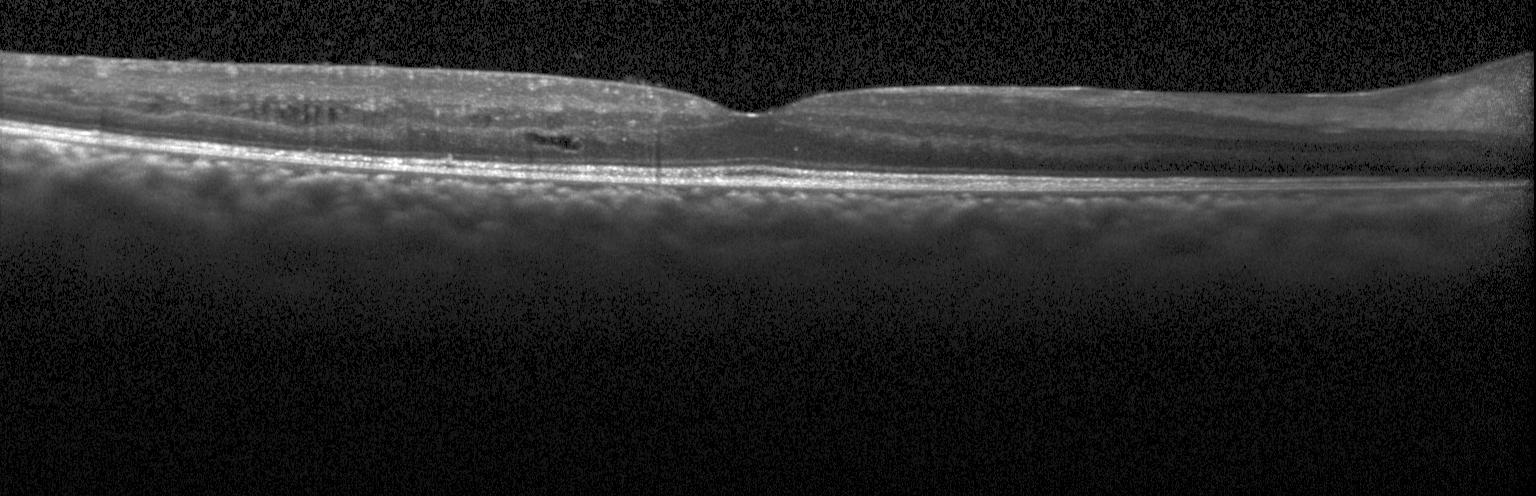
OCT scan showing diabetic macular edema.